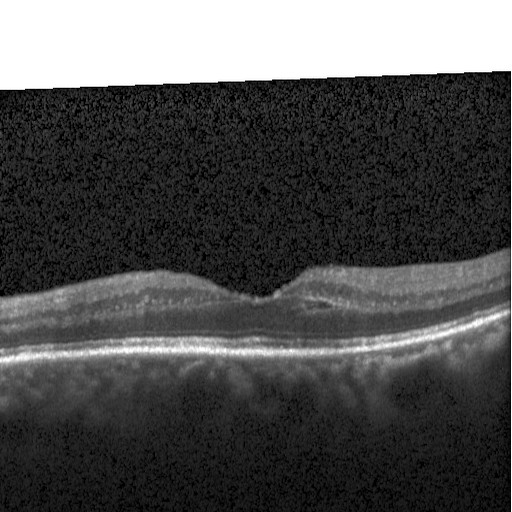

OCT line scan.
Diagnosis: diabetic macular edema (DME).